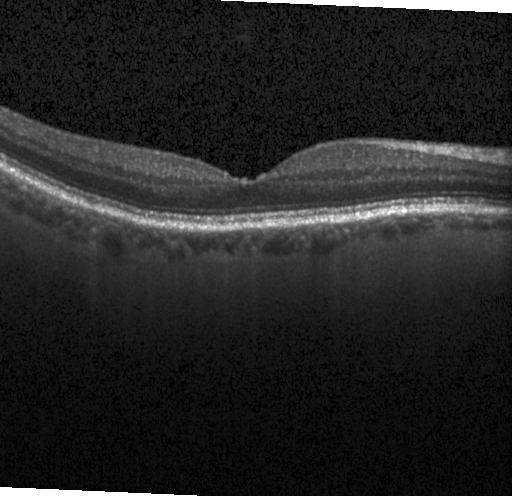
Optical coherence tomography B-scan; horizontal scan through the fovea; Heidelberg Spectralis; spectral-domain OCT.
Finding: neither CNV, DME, nor drusen.